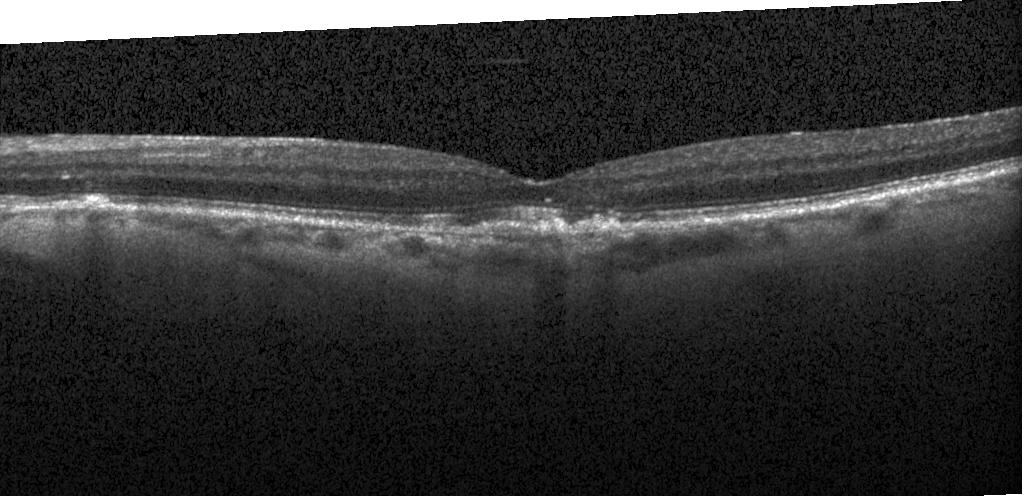 Retinal OCT cross-section; horizontal scan through the fovea
Diagnosis: a choroidal neovascular membrane.